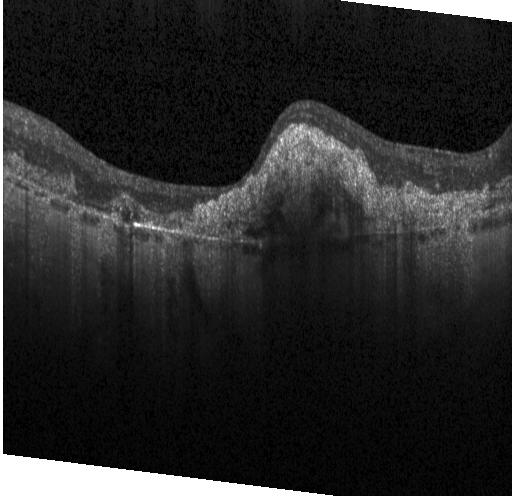
Spectral-domain OCT B-scan: a choroidal neovascular membrane.